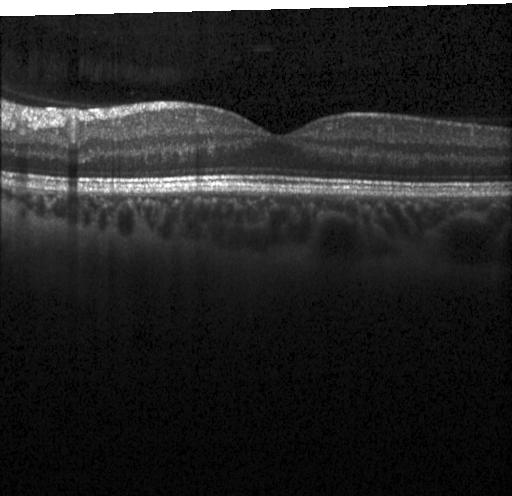
Instrument: Heidelberg Spectralis. SD-OCT. Horizontal scan through the fovea. Optical coherence tomography scan. No choroidal neovascularization, no diabetic macular edema, and no drusen.